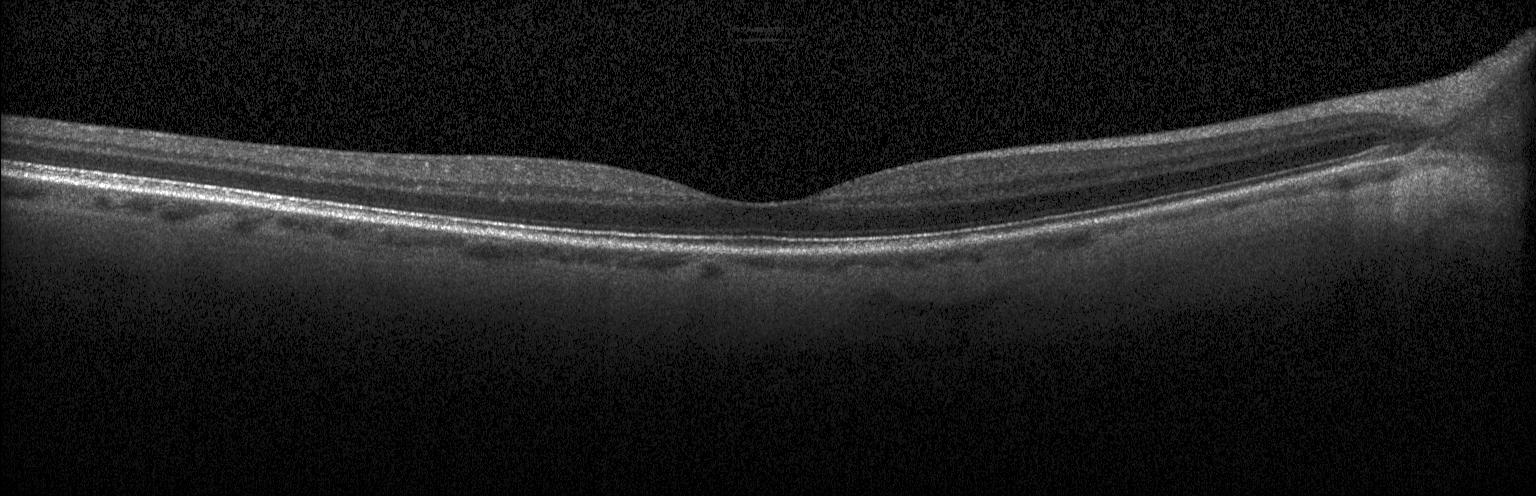

Assessment: neither choroidal neovascularization, diabetic macular edema, nor drusen.